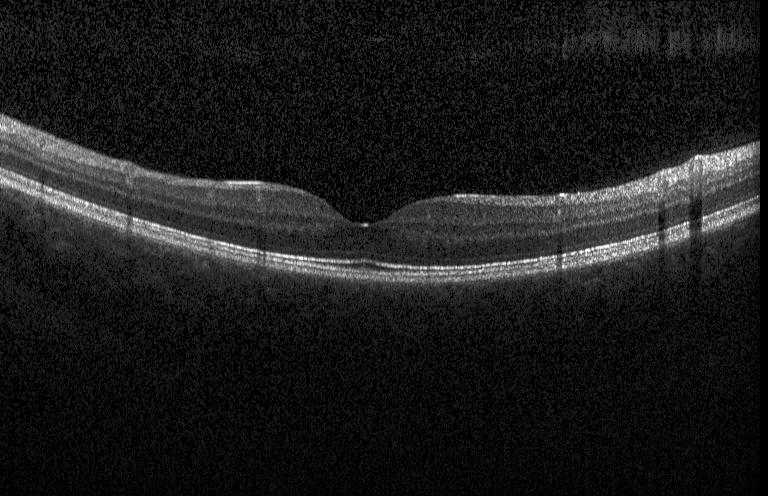
OCT B-scan; spectral-domain optical coherence tomography — Assessment: neither CNV, DME, nor drusen.